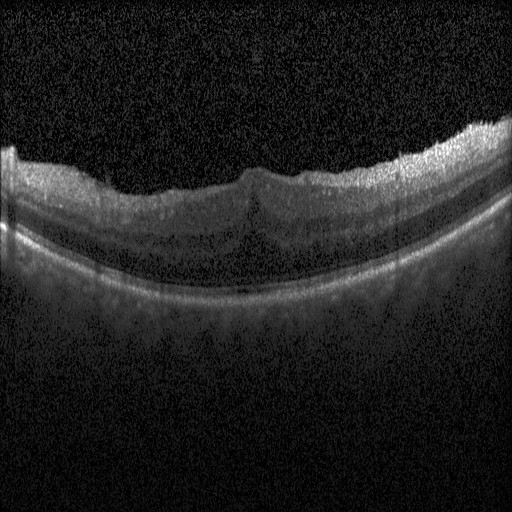
Optical coherence tomography scan. Impression: diabetic macular edema (DME).